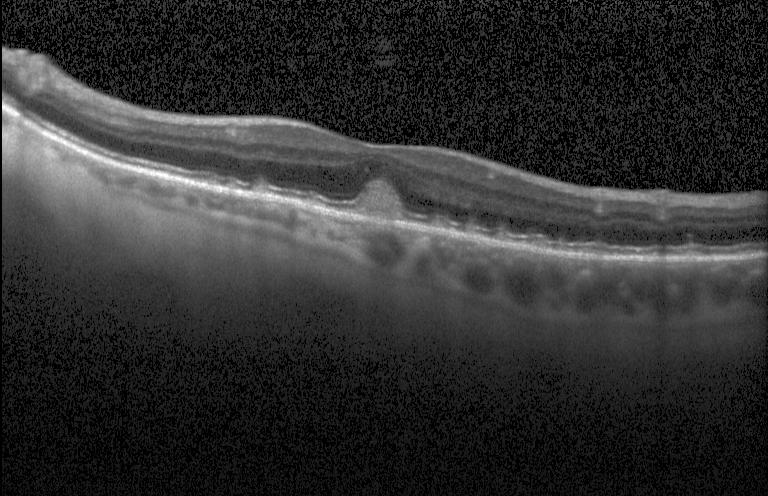
Impression: a choroidal neovascular membrane.